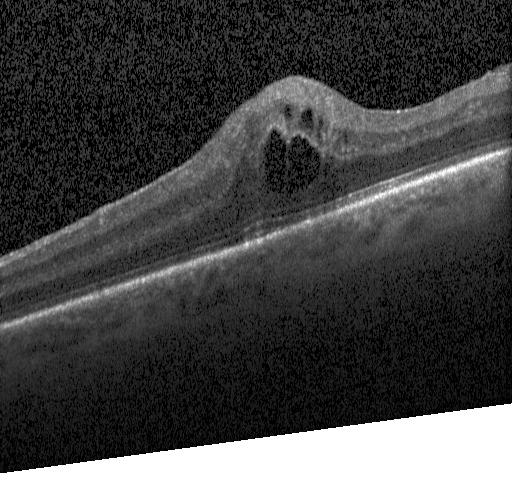
Horizontal scan through the fovea, retinal OCT B-scan, spectral-domain OCT, instrument: Heidelberg Spectralis — Diagnosis: DME.